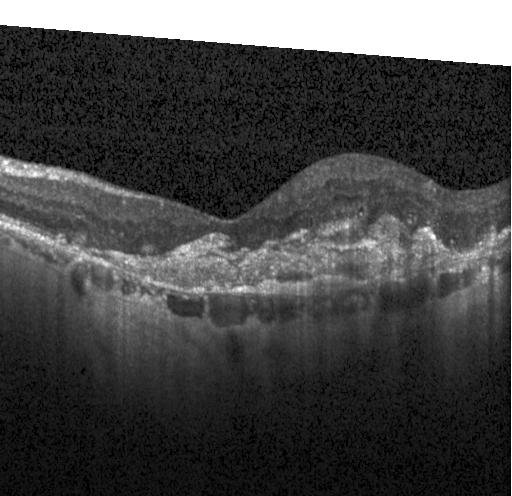 Horizontal scan through the fovea. OCT line scan
Finding: choroidal neovascularization (CNV).